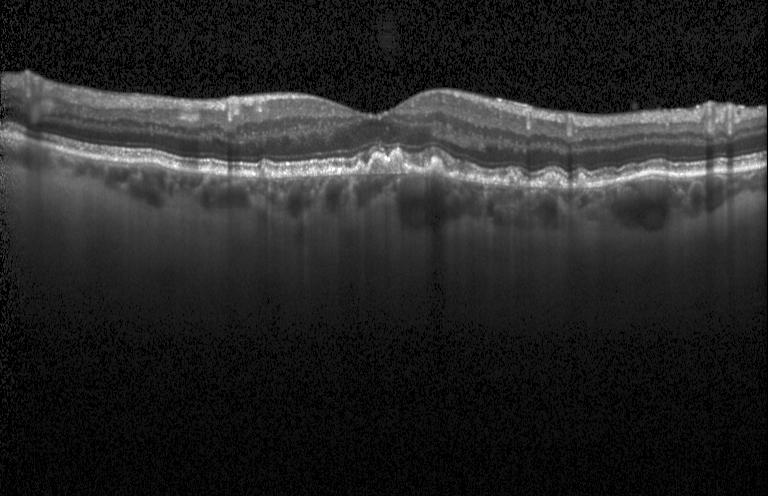
Optical coherence tomography B-scan, instrument: Heidelberg Spectralis, centered on the fovea, SD-OCT. Macular OCT: multiple drusen.